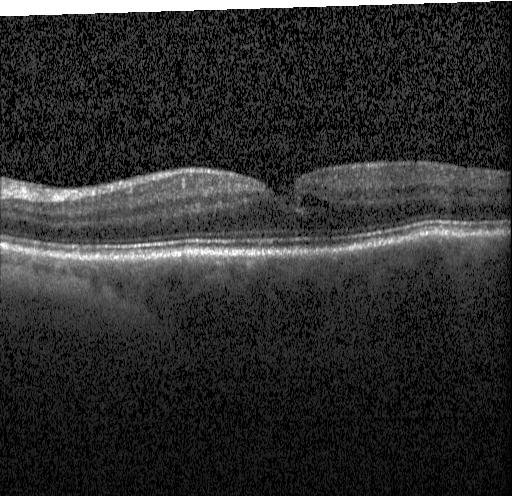
OCT B-scan; Heidelberg Spectralis OCT system; spectral-domain OCT. Impression: DME.